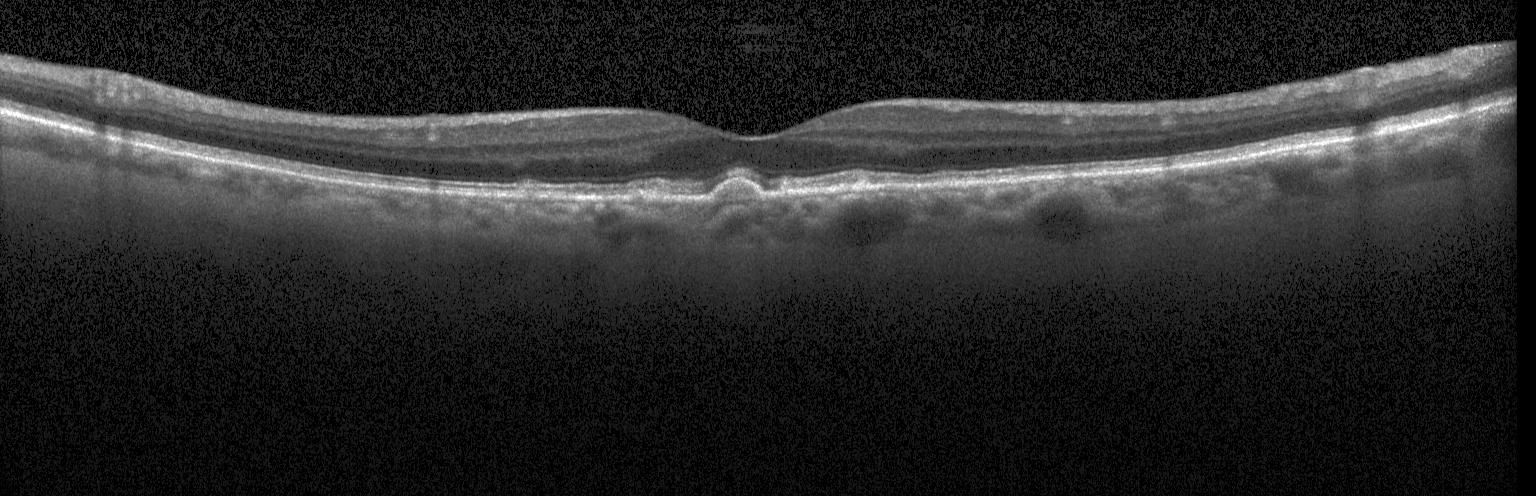
Heidelberg Spectralis OCT system, SD-OCT, fovea-centered, optical coherence tomography B-scan — Diagnosis: sub-RPE drusenoid deposits.